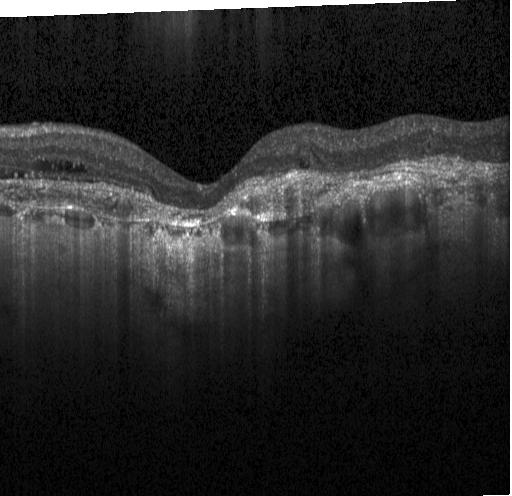

A choroidal neovascular membrane.